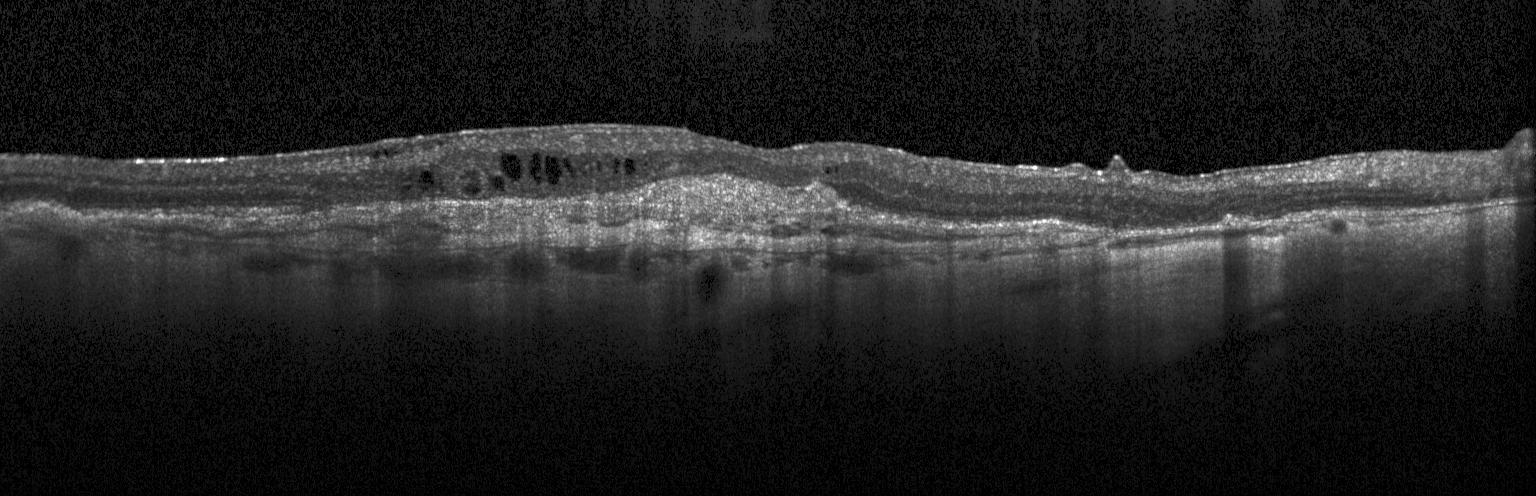
Instrument: Heidelberg Spectralis, OCT line scan — Choroidal neovascularization (CNV).